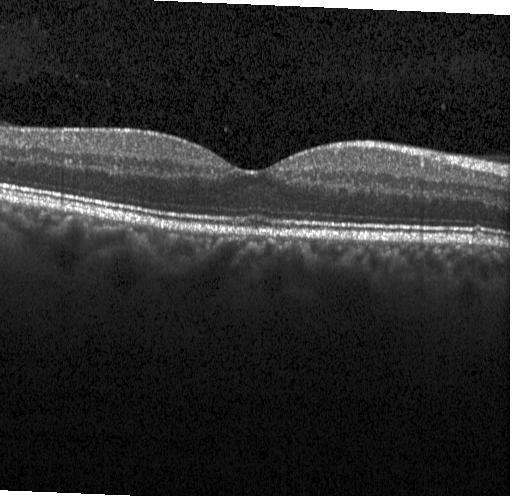
The scan shows neither CNV, DME, nor drusen.